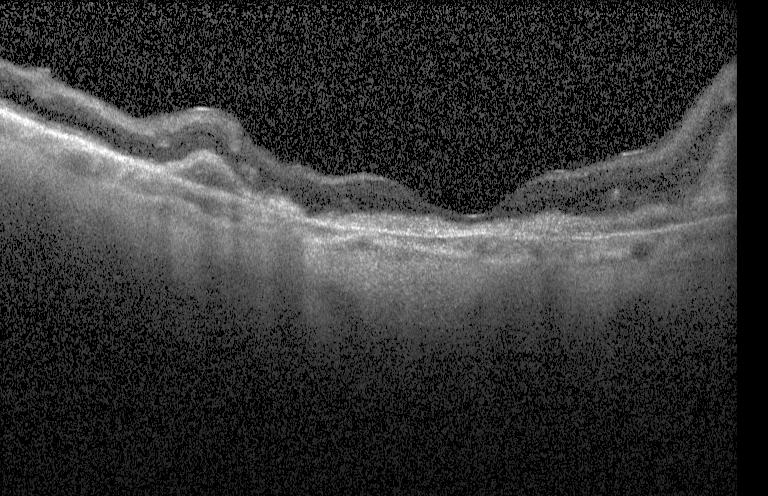 Spectral-domain OCT; retinal OCT cross-section; centered on the fovea.
Macular OCT: CNV.